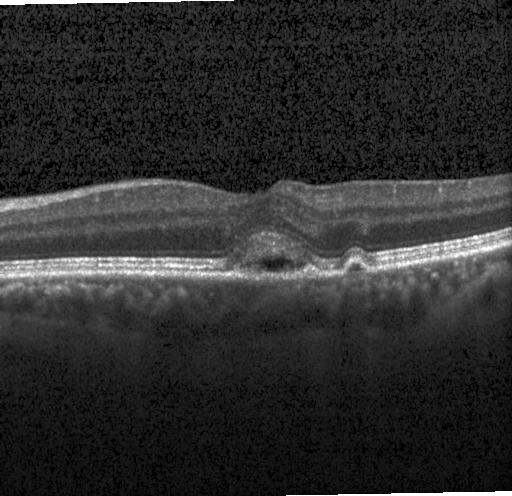

Finding: a choroidal neovascular membrane.